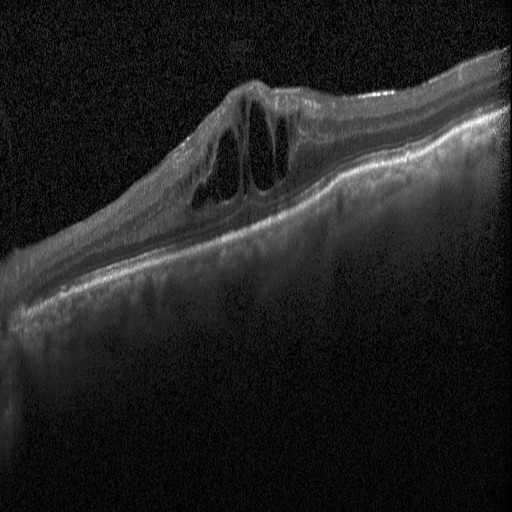 Retinal OCT B-scan. Impression: diabetic macular edema.